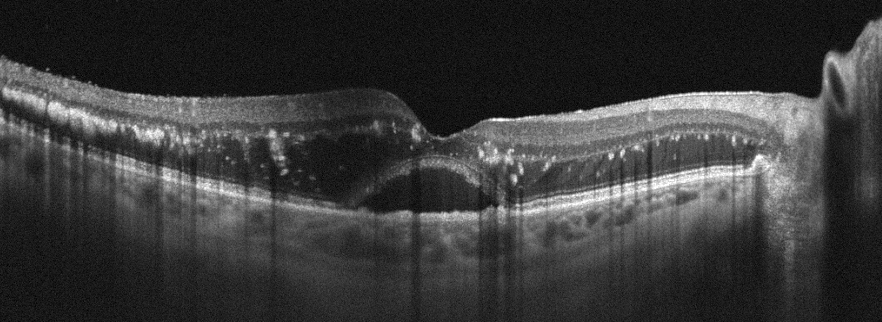
Right eye · OCT B-scan.
Retinal vein occlusion (RVO).